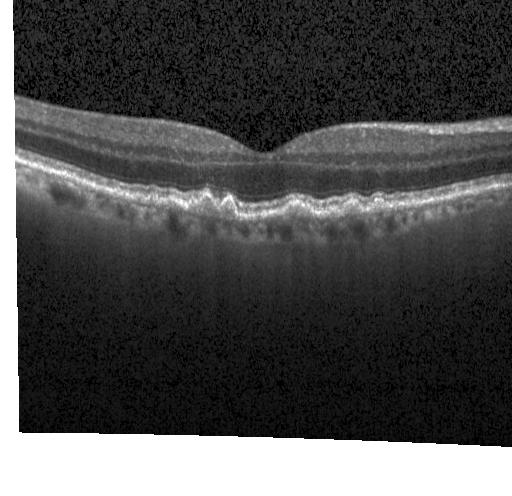
Retinal OCT cross-section. Diagnosis: sub-RPE drusenoid deposits.